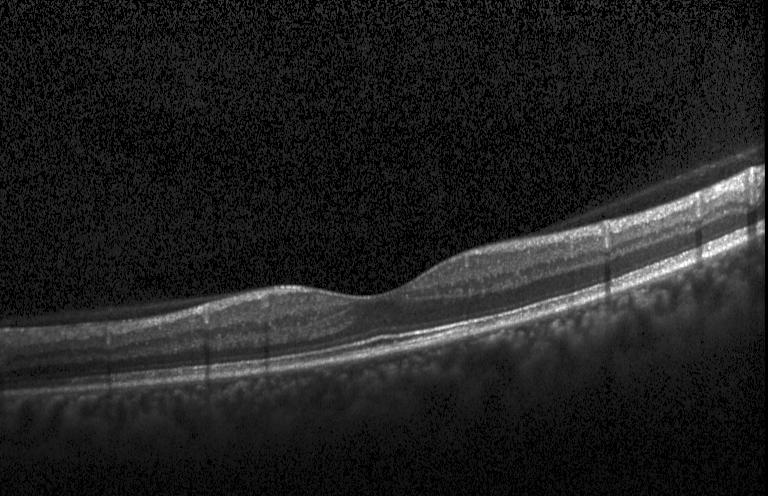
Spectral-domain OCT; acquired on a Heidelberg Spectralis; fovea-centered; OCT B-scan — Impression: neither choroidal neovascularization, diabetic macular edema, nor drusen.